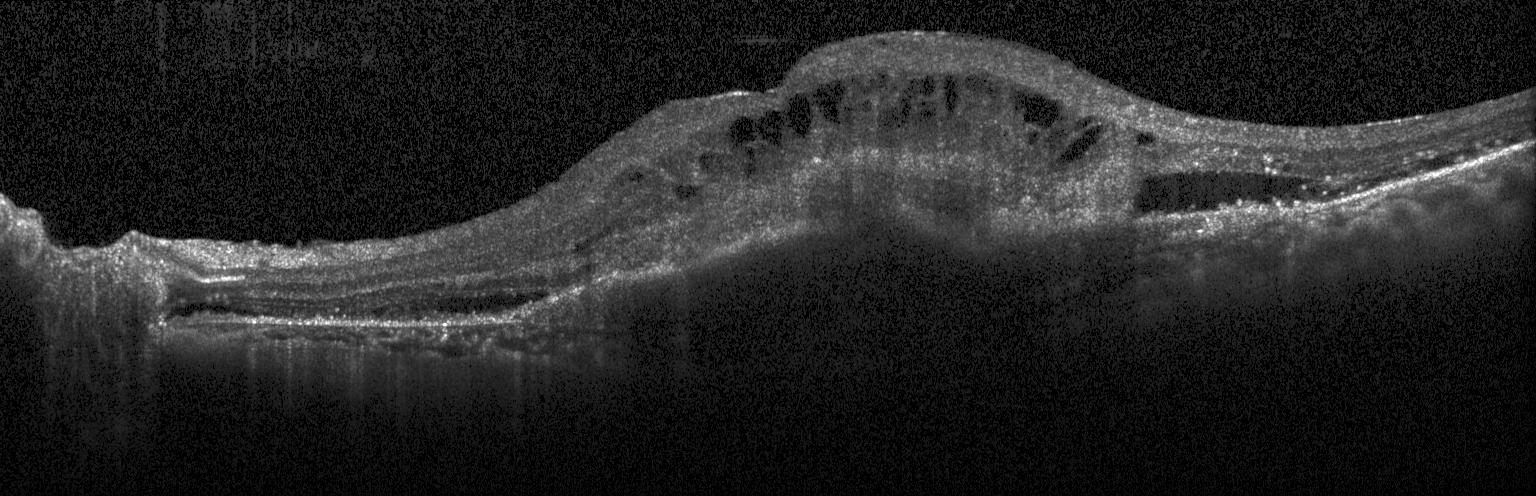 Retinal OCT B-scan.
Macular OCT: CNV.